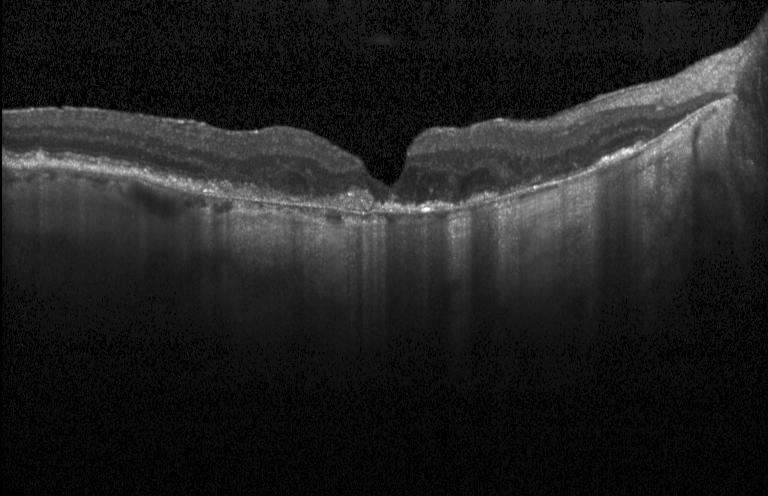

Diagnosis: a choroidal neovascular membrane.